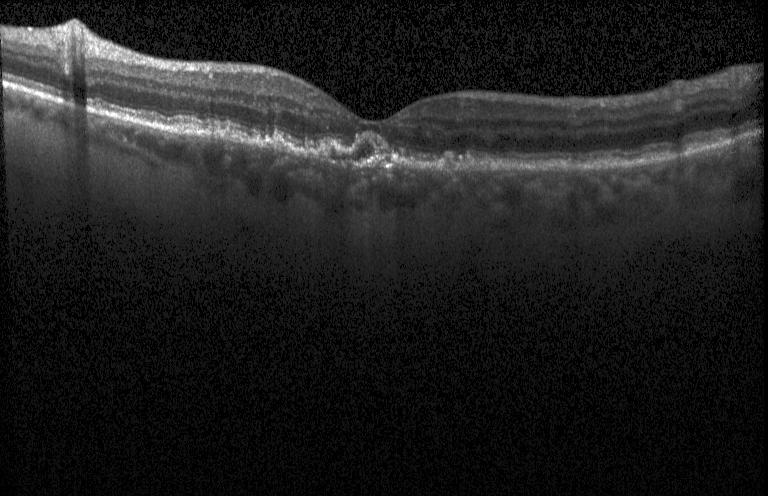
Instrument: Heidelberg Spectralis · retinal OCT B-scan · horizontal scan through the fovea
Assessment: a choroidal neovascular membrane.